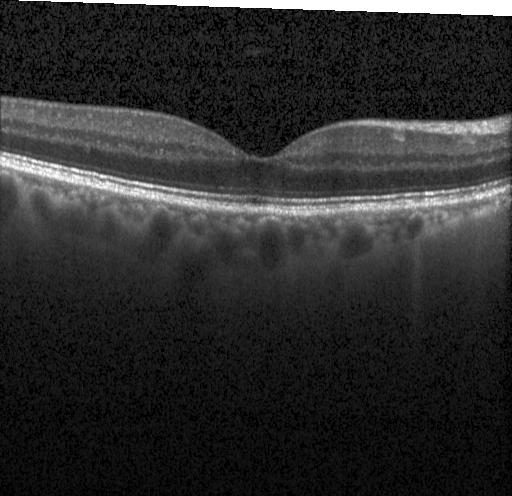 Impression: neither choroidal neovascularization, diabetic macular edema, nor drusen.